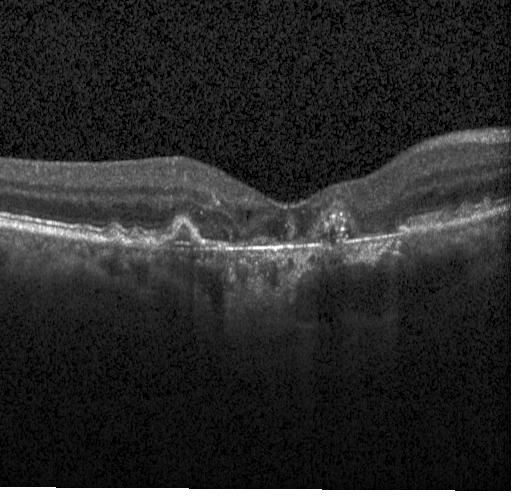

Spectral-domain OCT B-scan: a choroidal neovascular membrane.